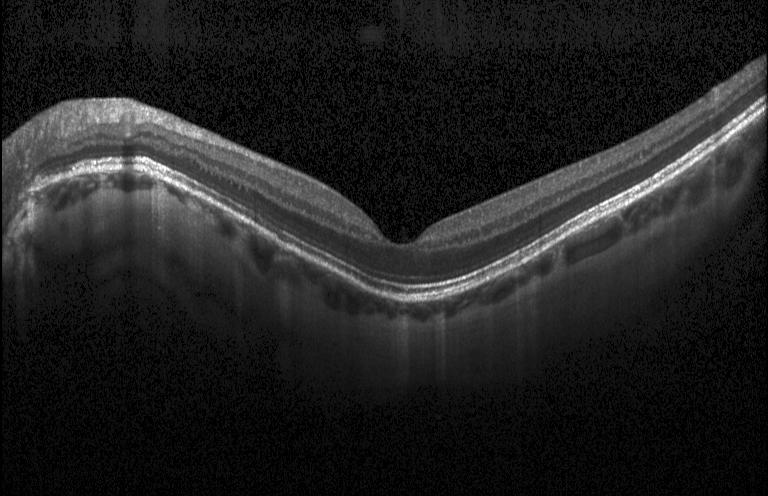

Finding: neither choroidal neovascularization, diabetic macular edema, nor drusen.